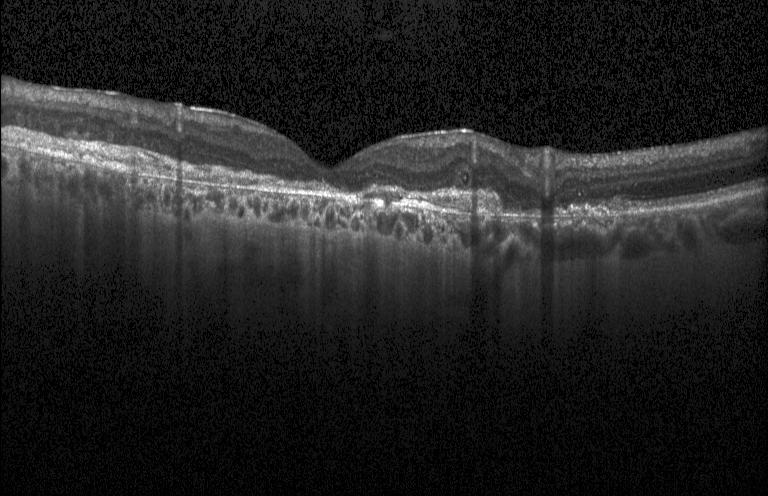 Optical coherence tomography scan. Impression: CNV.